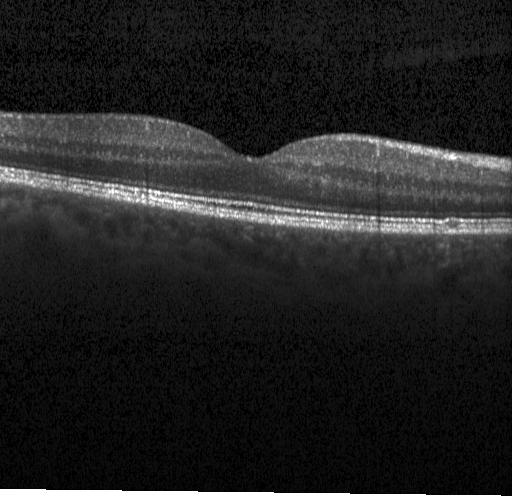 Macular scan · instrument: Heidelberg Spectralis · optical coherence tomography scan · spectral-domain optical coherence tomography
Impression: no evidence of choroidal neovascularization, diabetic macular edema, or drusen.